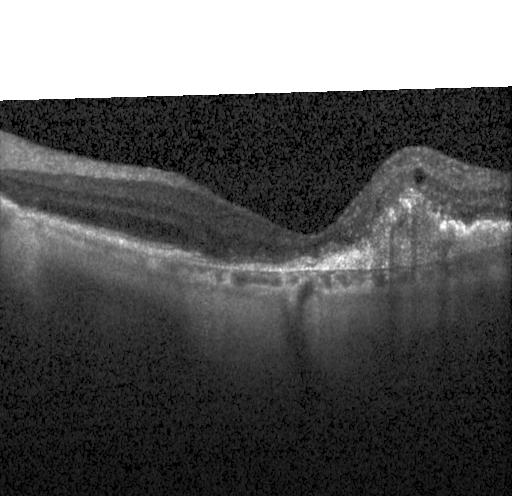
Horizontal scan through the fovea. Spectral-domain optical coherence tomography. Optical coherence tomography scan.
Finding: a choroidal neovascular membrane.